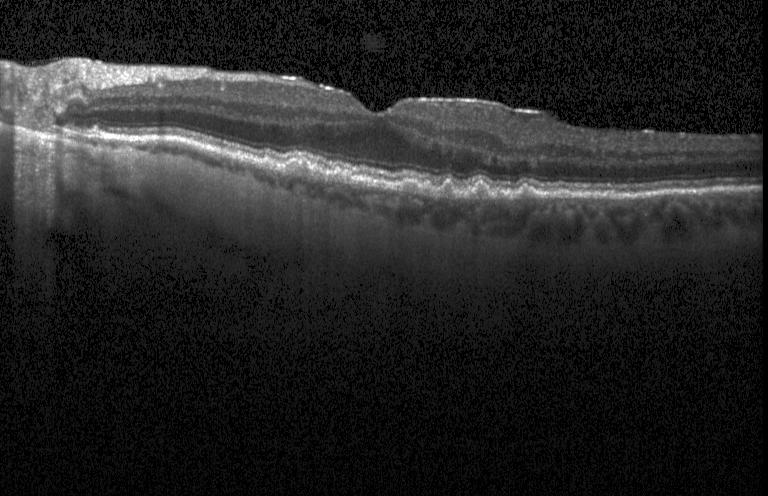

Macular OCT demonstrating drusen.